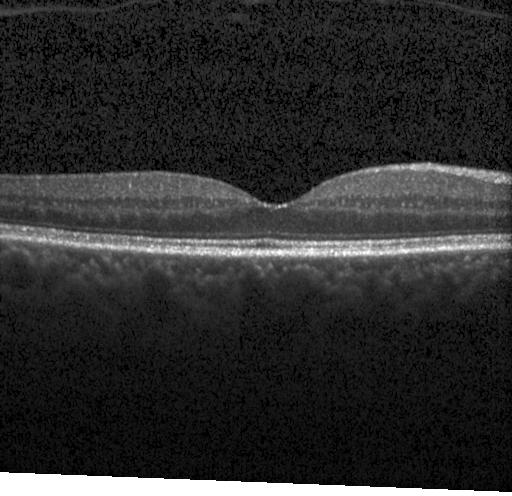

Optical coherence tomography scan · spectral-domain OCT — OCT finding: no evidence of choroidal neovascularization, diabetic macular edema, or drusen.